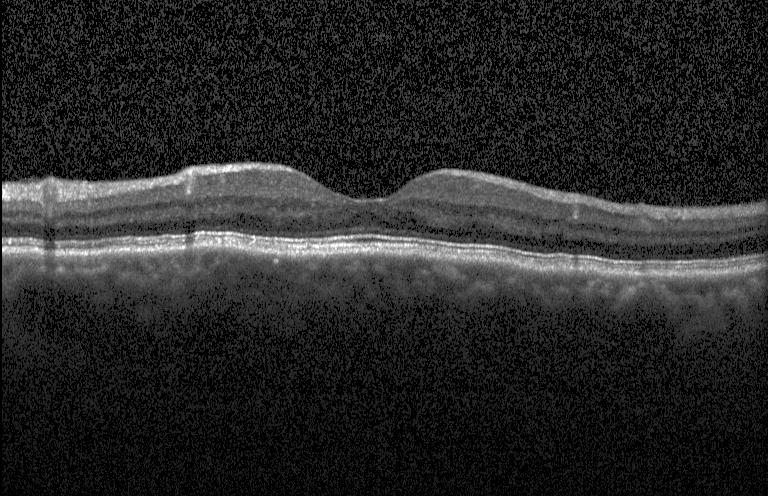
Optical coherence tomography scan. Impression: neither choroidal neovascularization, diabetic macular edema, nor drusen.